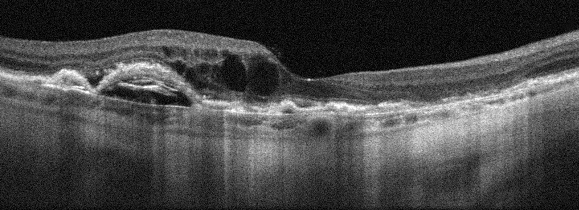
Retinal OCT B-scan · right eye
AMD.